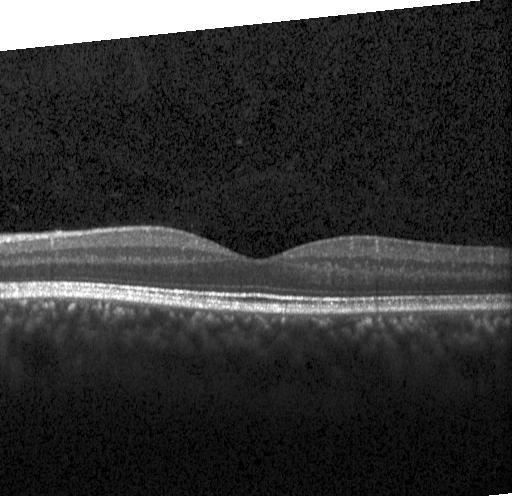 Retinal OCT B-scan · spectral-domain optical coherence tomography · Heidelberg Spectralis.
Finding: no choroidal neovascularization, diabetic macular edema, or drusen.